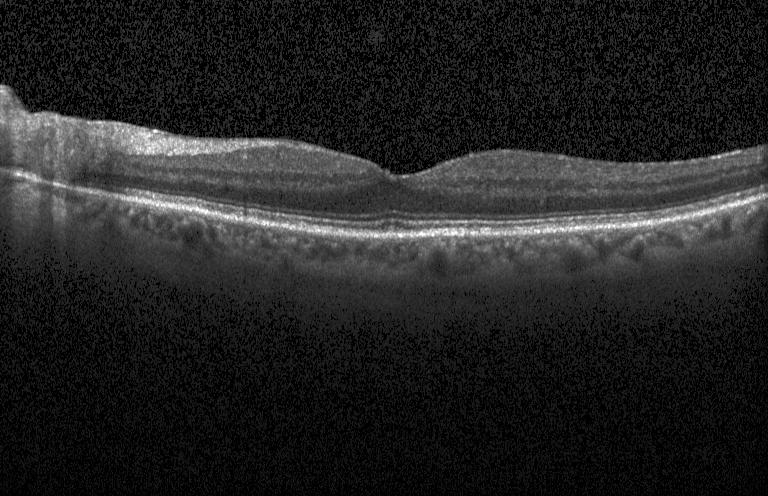
Spectral-domain OCT. Retinal OCT B-scan. No choroidal neovascularization, diabetic macular edema, or drusen.